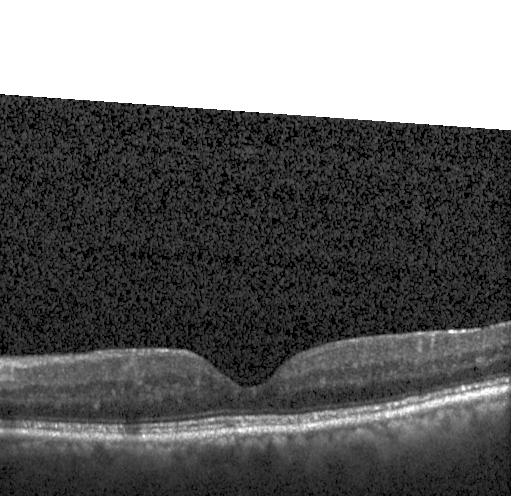
Diagnosis: no choroidal neovascularization, no diabetic macular edema, and no drusen.